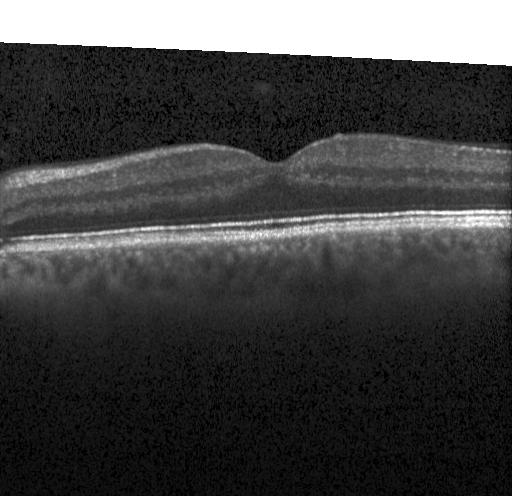

OCT line scan
Impression: no choroidal neovascularization, no diabetic macular edema, and no drusen.